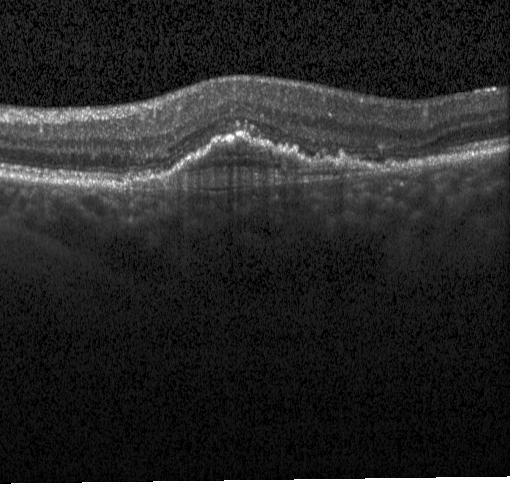

Optical coherence tomography scan.
Dx: choroidal neovascularization (CNV).